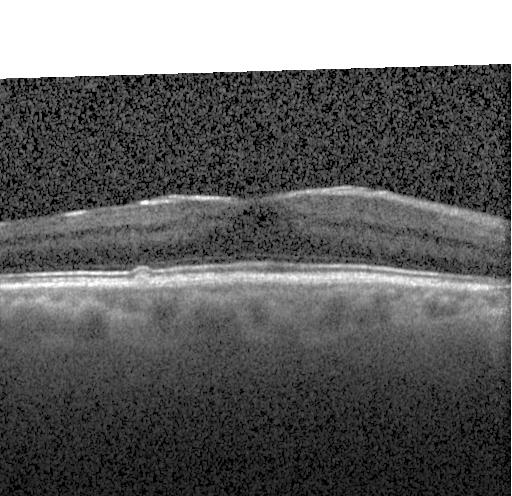 Impression: multiple drusen.